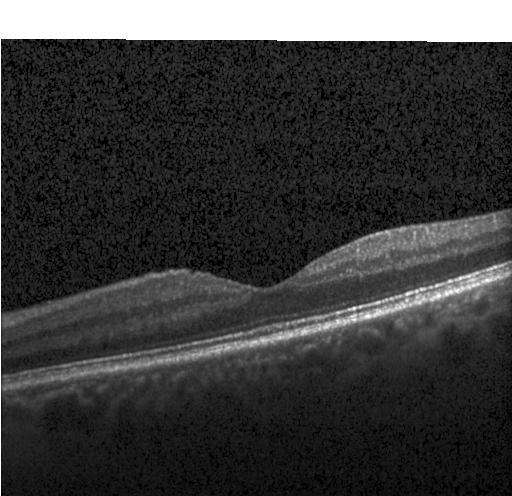 Finding: neither choroidal neovascularization, diabetic macular edema, nor drusen.